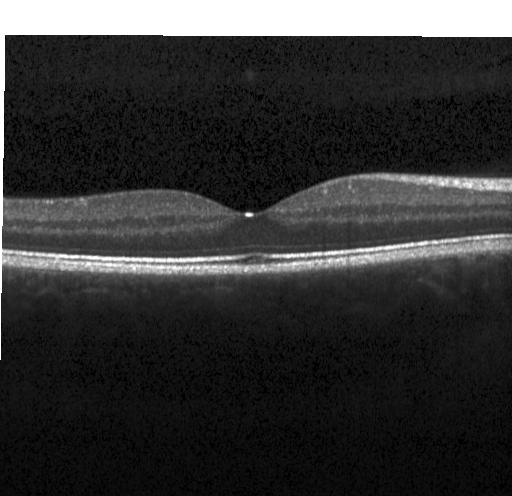

Through the macula, retinal OCT cross-section, spectral-domain optical coherence tomography, Heidelberg Spectralis OCT system
Diagnosis: no choroidal neovascularization, diabetic macular edema, or drusen.